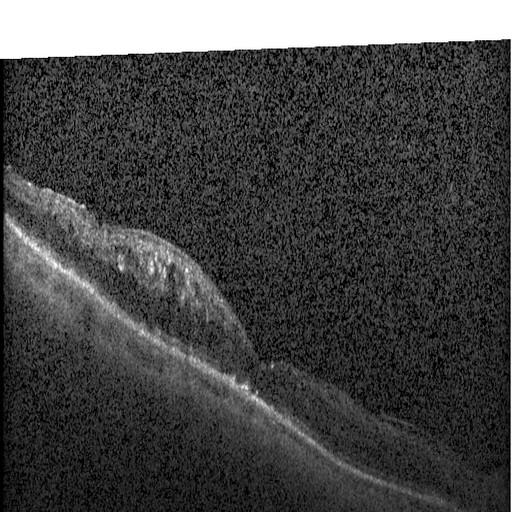 Fovea-centered; SD-OCT; optical coherence tomography scan
Impression: diabetic macular edema.